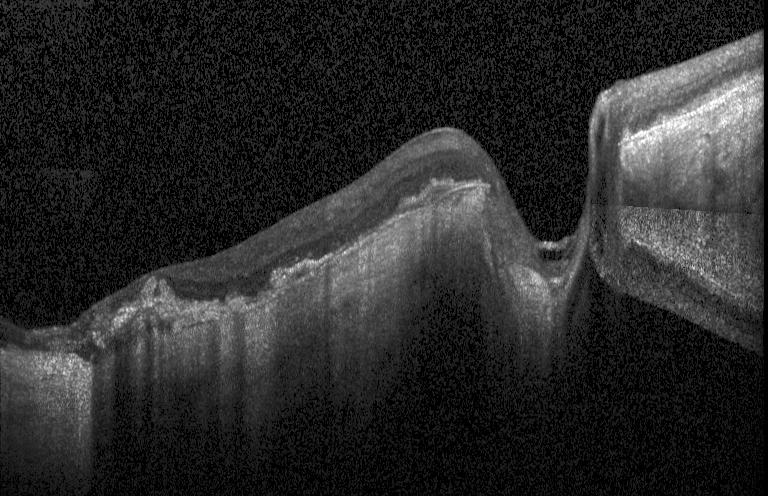 This B-scan demonstrates a choroidal neovascular membrane.